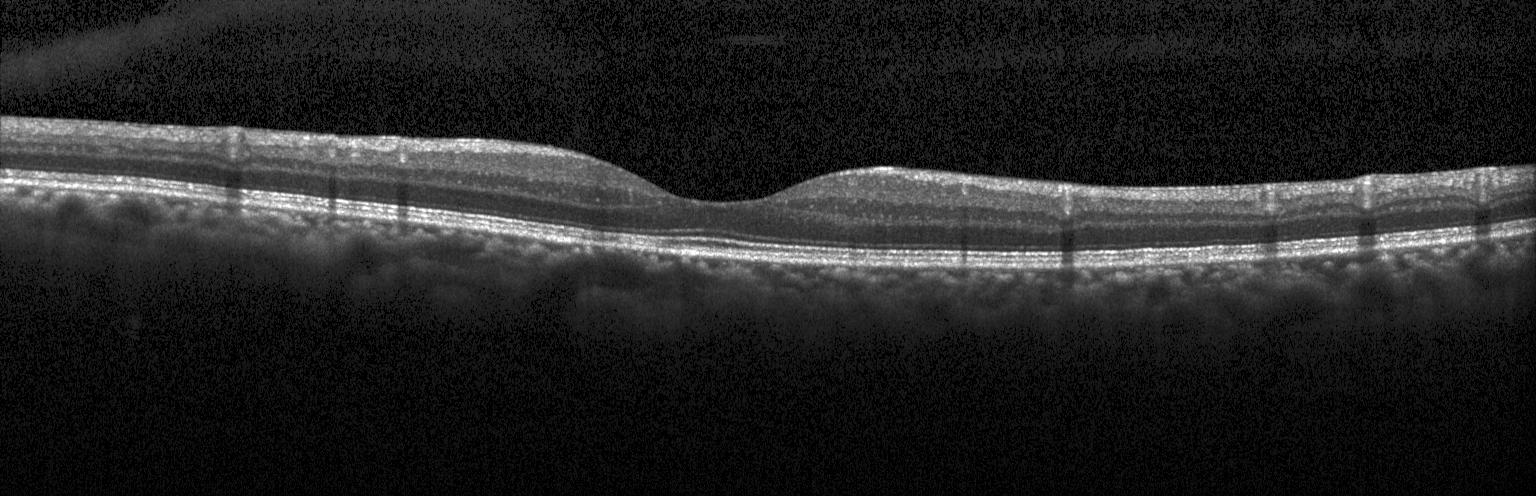
Spectral-domain OCT B-scan: neither choroidal neovascularization, diabetic macular edema, nor drusen.